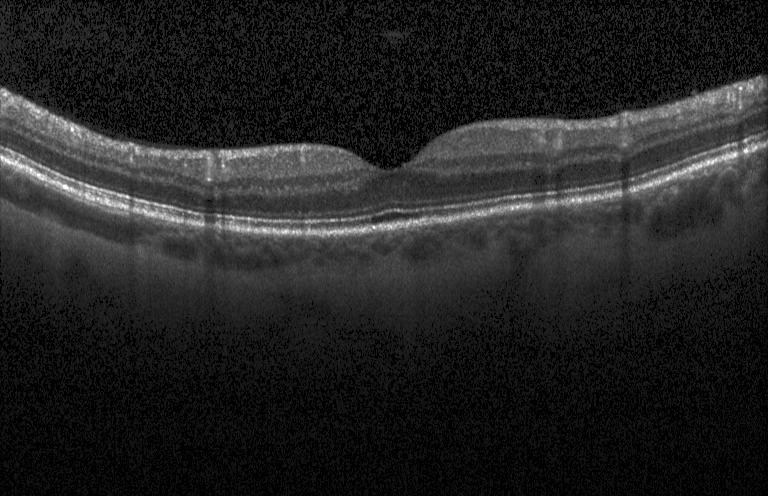

Through the macula. Optical coherence tomography scan
Finding: neither choroidal neovascularization, diabetic macular edema, nor drusen.